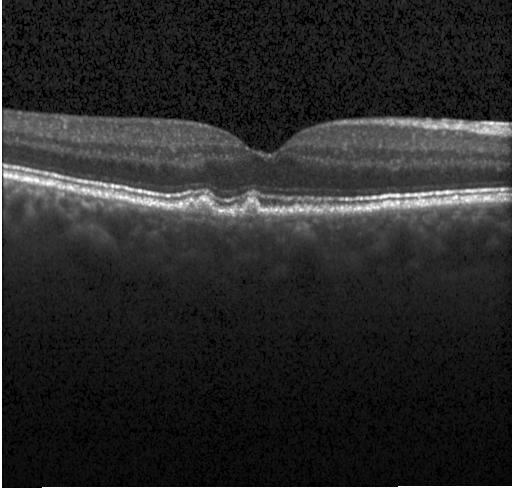
Through the macula. Heidelberg Spectralis OCT system. Retinal OCT cross-section.
Macular OCT: drusen.